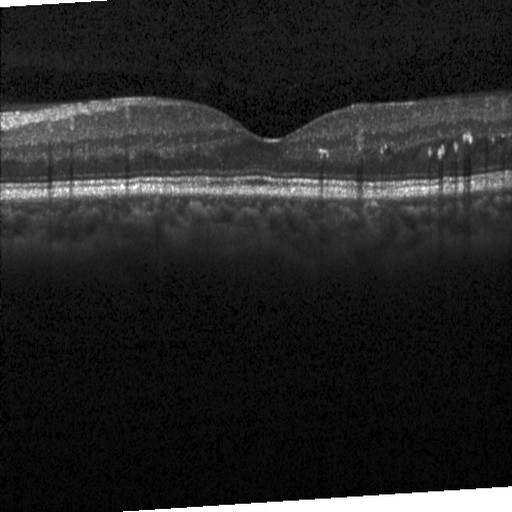
OCT line scan — Finding: diabetic macular edema.